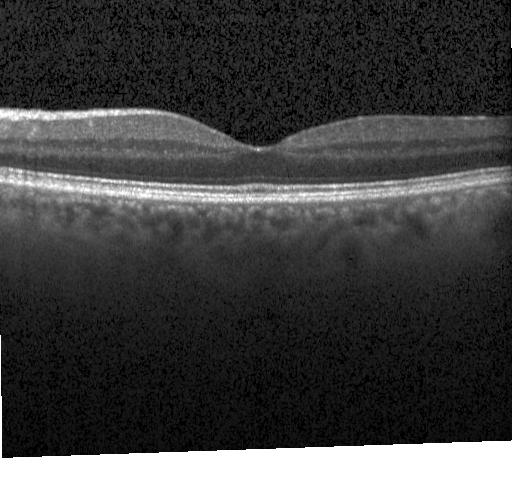

Impression: neither CNV, DME, nor drusen.